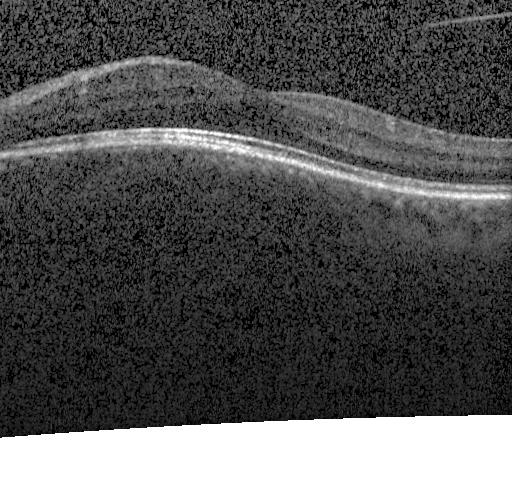
Retinal OCT cross-section. Spectral-domain optical coherence tomography. Through the macula. Heidelberg Spectralis OCT system.
Macular OCT: no choroidal neovascularization, diabetic macular edema, or drusen.